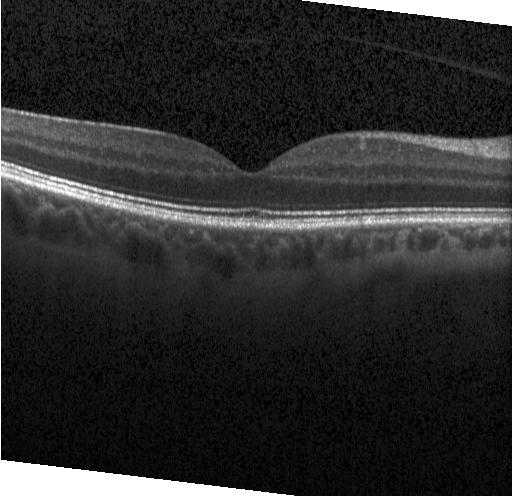

Optical coherence tomography B-scan. No choroidal neovascularization, diabetic macular edema, or drusen.